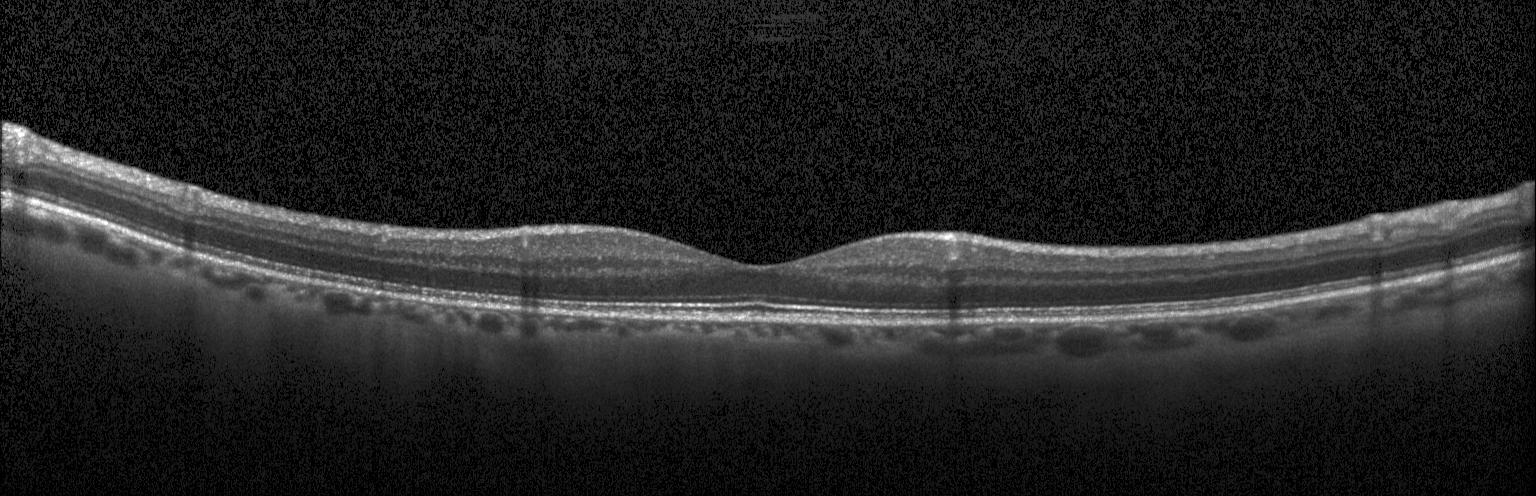 Spectral-domain OCT · fovea-centered · acquired on a Heidelberg Spectralis · optical coherence tomography scan — The scan shows neither CNV, DME, nor drusen.